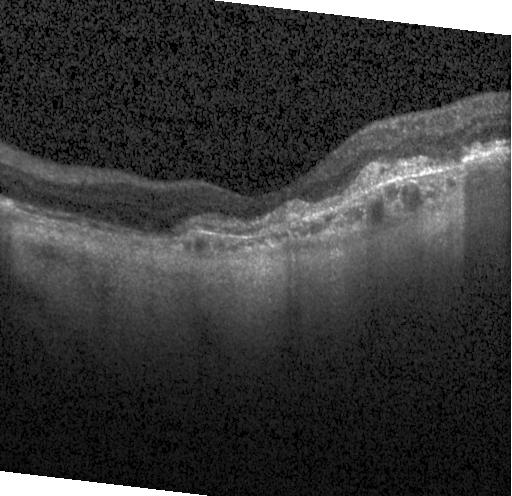
Optical coherence tomography scan
Diagnosis: choroidal neovascularization (CNV).